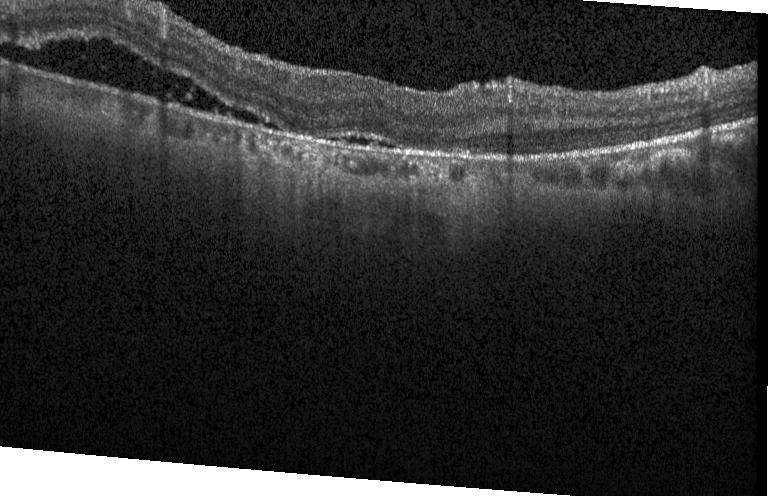
Diagnosis: a choroidal neovascular membrane.